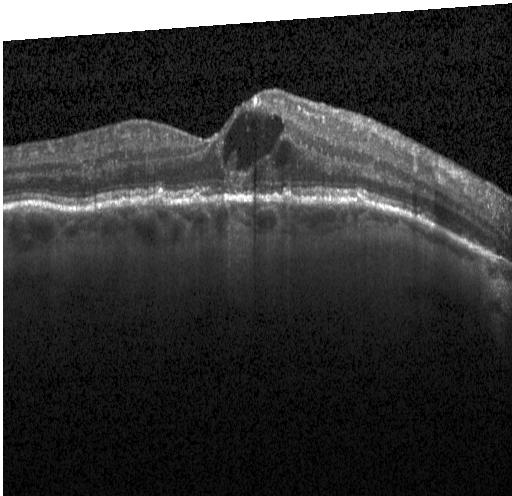

Assessment: choroidal neovascularization.